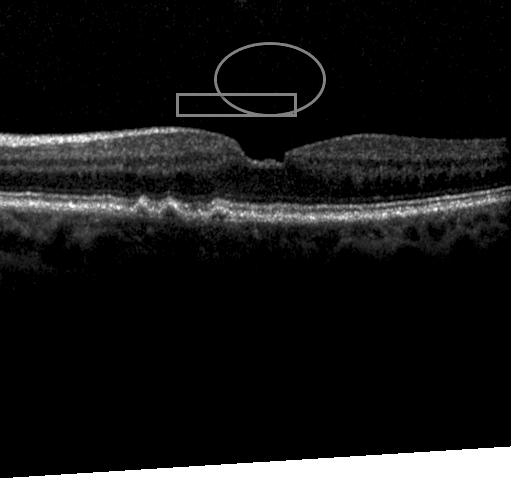
Impression: multiple drusen.